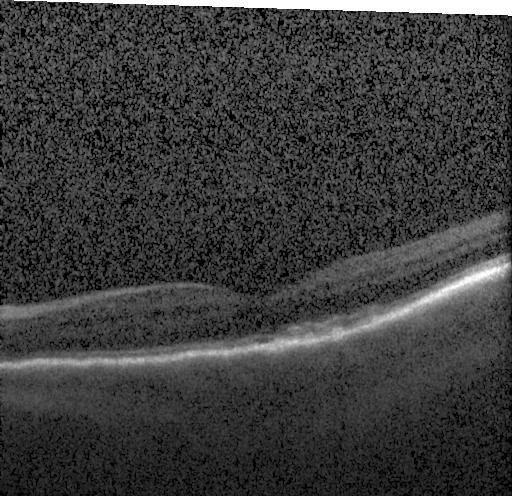
OCT B-scan showing sub-RPE drusenoid deposits.